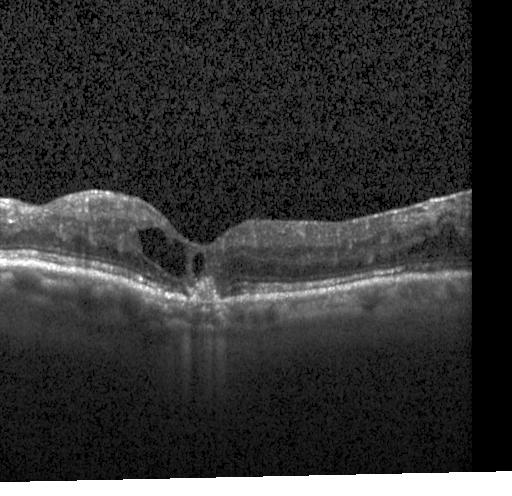 OCT B-scan · SD-OCT · Heidelberg Spectralis · fovea-centered. This B-scan demonstrates choroidal neovascularization (CNV).